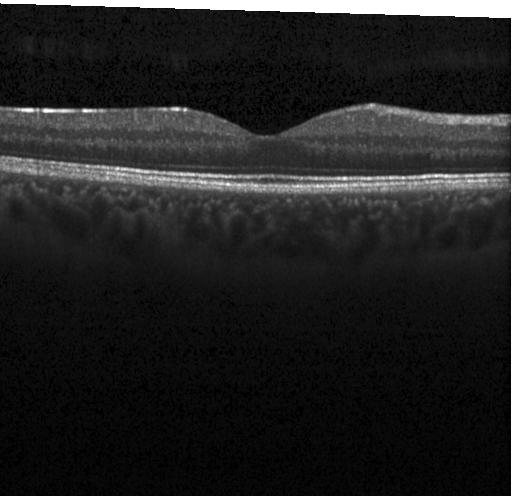 Impression: no CNV, no DME, and no drusen.